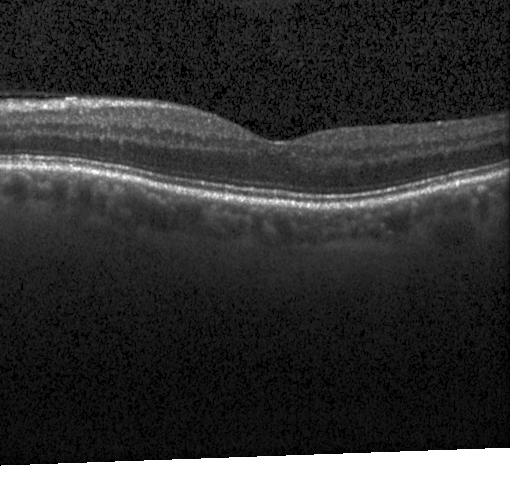 Macular scan, OCT line scan
Impression: no CNV, no DME, and no drusen.